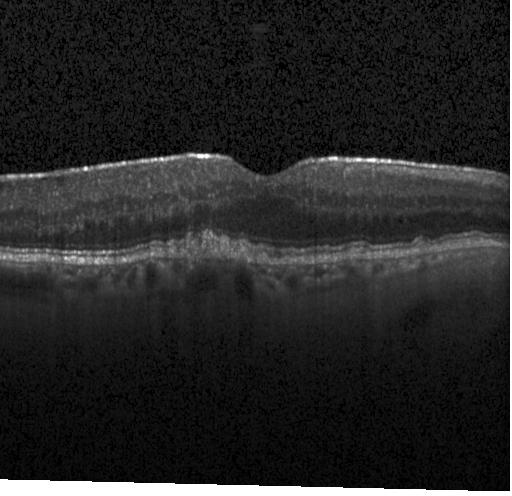 Spectral-domain OCT B-scan: drusen.